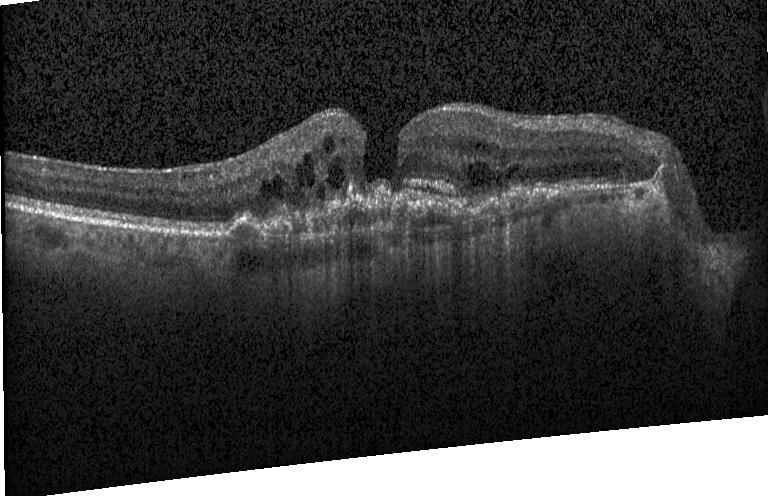
Heidelberg Spectralis OCT system · retinal OCT B-scan · macular scan
CNV.